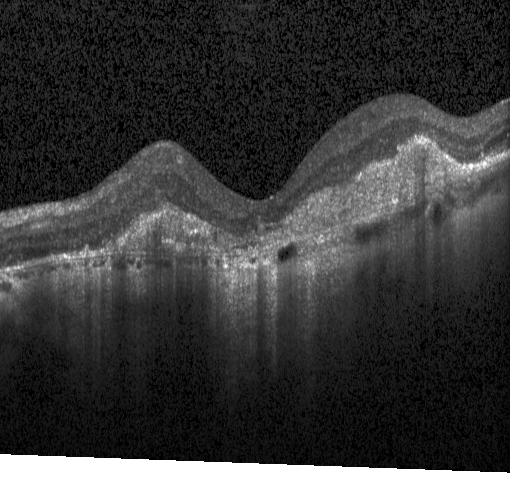 Spectral-domain OCT; through the macula; Heidelberg Spectralis OCT system; optical coherence tomography B-scan. The scan shows a choroidal neovascular membrane.